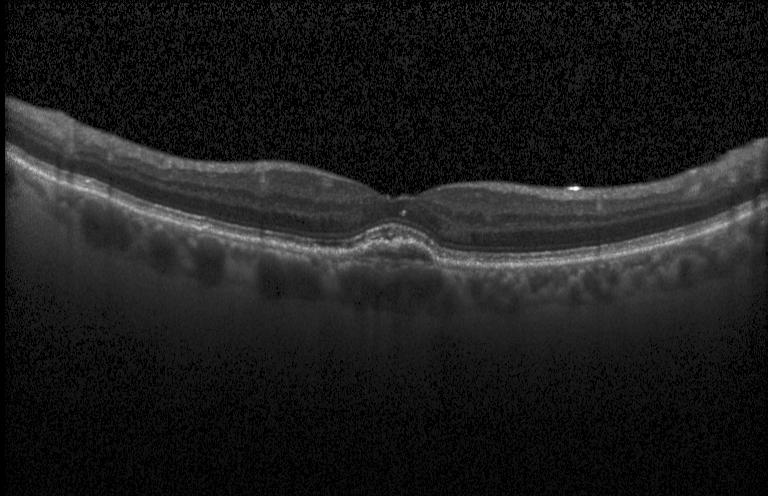
Retinal OCT cross-section · centered on the fovea · acquired on a Heidelberg Spectralis. Choroidal neovascularization (CNV).